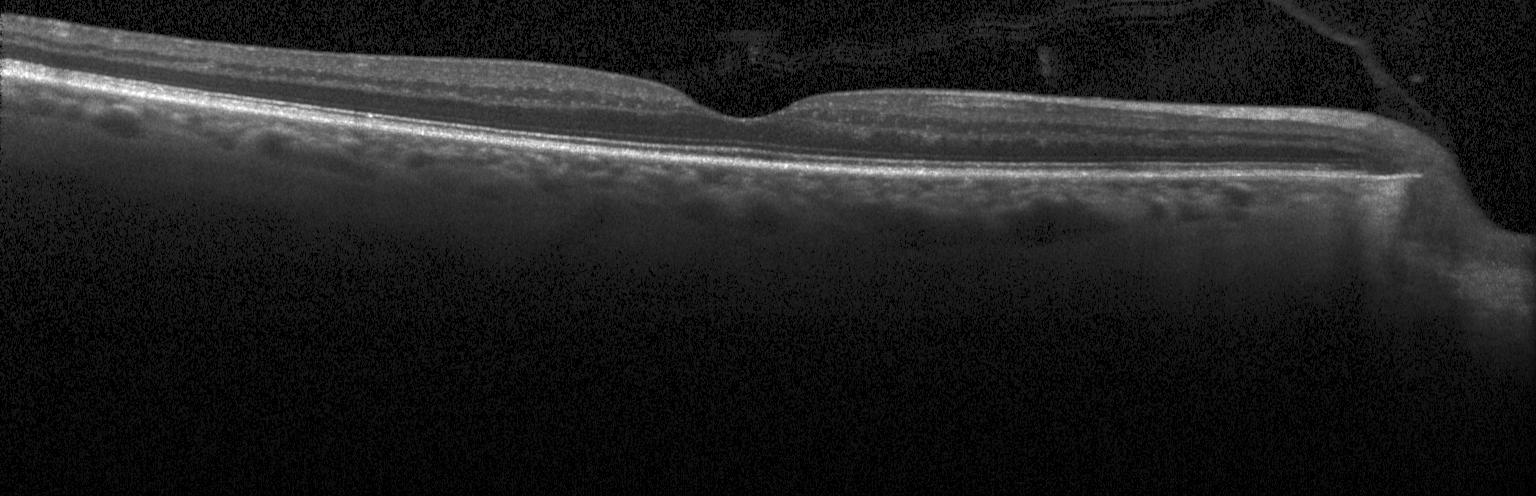
Retinal OCT B-scan
Assessment: no evidence of CNV, DME, or drusen.